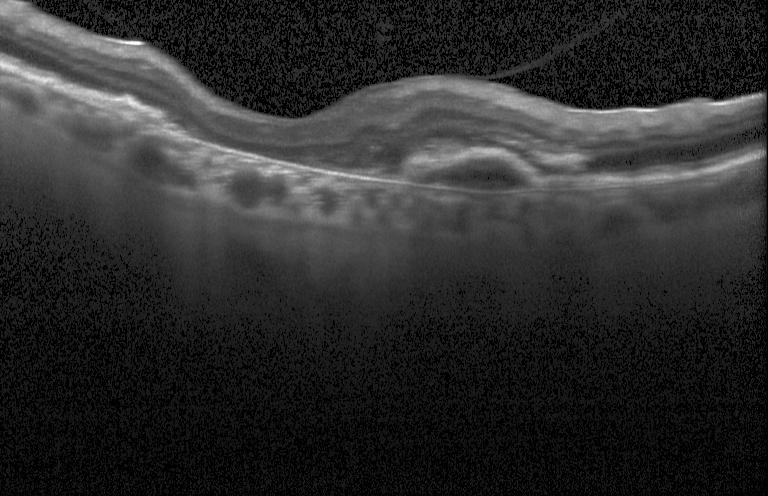 OCT B-scan. Heidelberg Spectralis OCT system. Macular scan — Finding: a choroidal neovascular membrane.